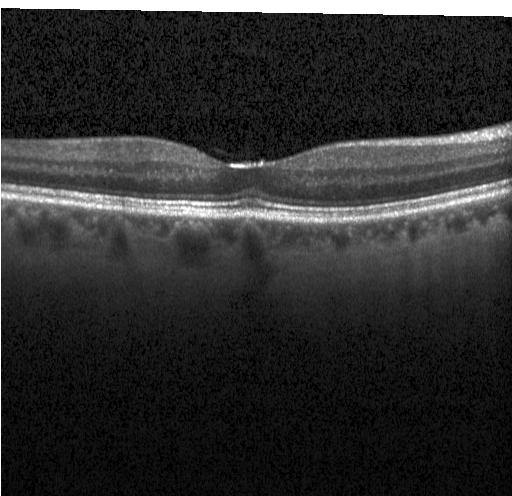 Through the macula. Heidelberg Spectralis. Optical coherence tomography B-scan
Finding: no choroidal neovascularization, no diabetic macular edema, and no drusen.